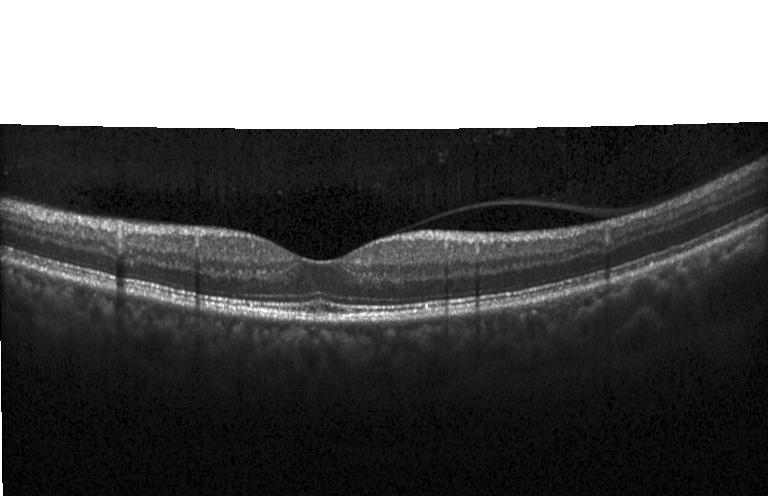
Retinal OCT cross-section, fovea-centered, acquired on a Heidelberg Spectralis, SD-OCT
Diagnosis: no evidence of choroidal neovascularization, diabetic macular edema, or drusen.